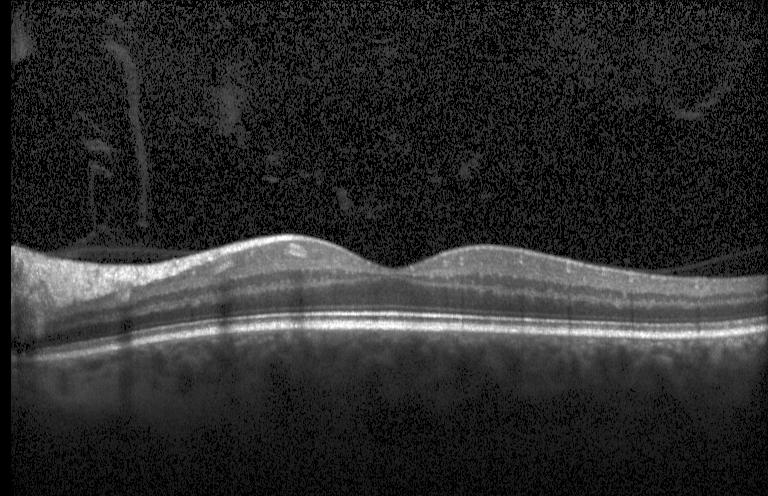 Impression: no evidence of choroidal neovascularization, diabetic macular edema, or drusen.